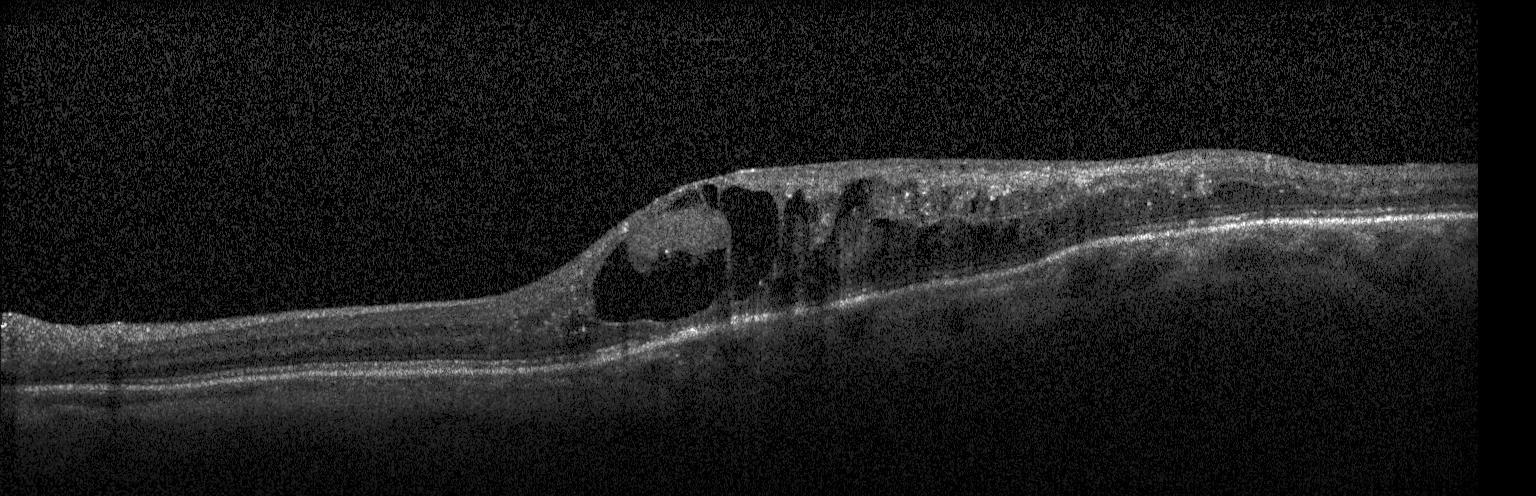 Impression: DME.